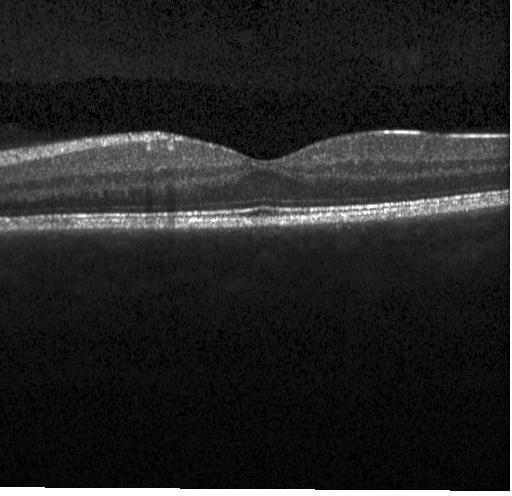 Spectral-domain optical coherence tomography. Through the macula. Retinal OCT cross-section — Assessment: no choroidal neovascularization, diabetic macular edema, or drusen.